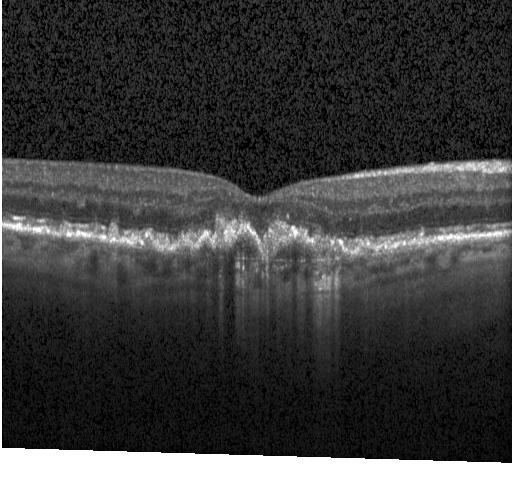 Horizontal scan through the fovea, OCT B-scan, instrument: Heidelberg Spectralis, spectral-domain OCT — Assessment: choroidal neovascularization.